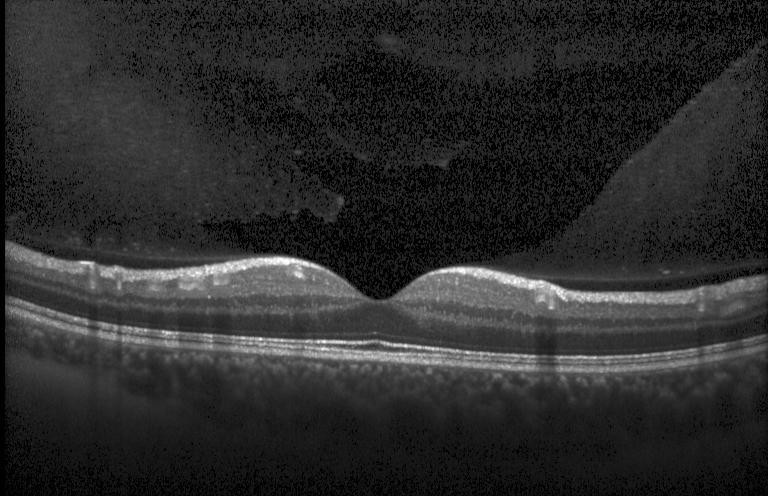
Spectral-domain optical coherence tomography · retinal OCT B-scan · horizontal scan through the fovea · instrument: Heidelberg Spectralis
Macular OCT: no evidence of choroidal neovascularization, diabetic macular edema, or drusen.